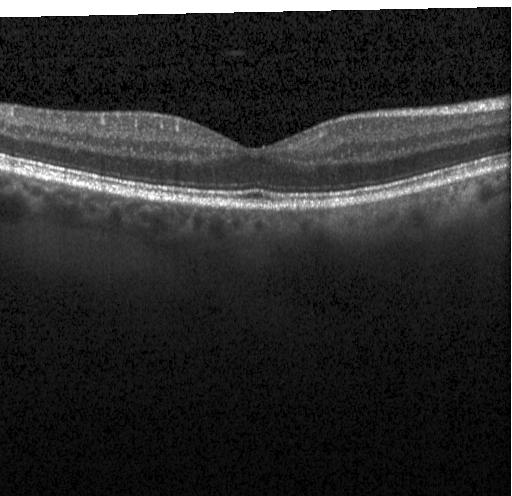
Centered on the fovea, Heidelberg Spectralis OCT system, spectral-domain OCT, OCT line scan.
Diagnosis: neither choroidal neovascularization, diabetic macular edema, nor drusen.